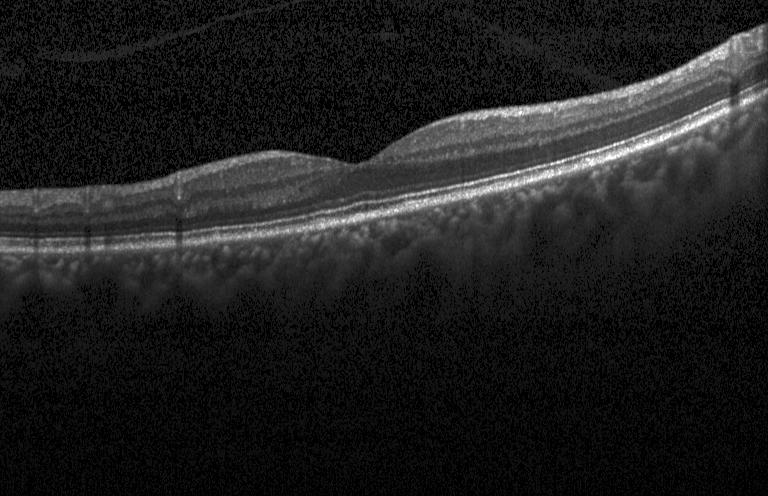 OCT line scan — Dx: no evidence of CNV, DME, or drusen.